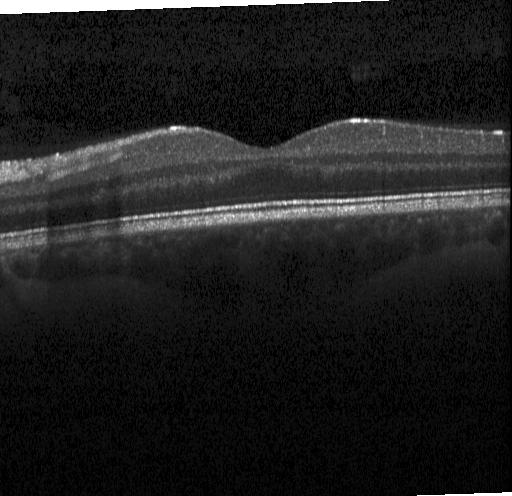
Optical coherence tomography scan; macular scan
Impression: no evidence of choroidal neovascularization, diabetic macular edema, or drusen.